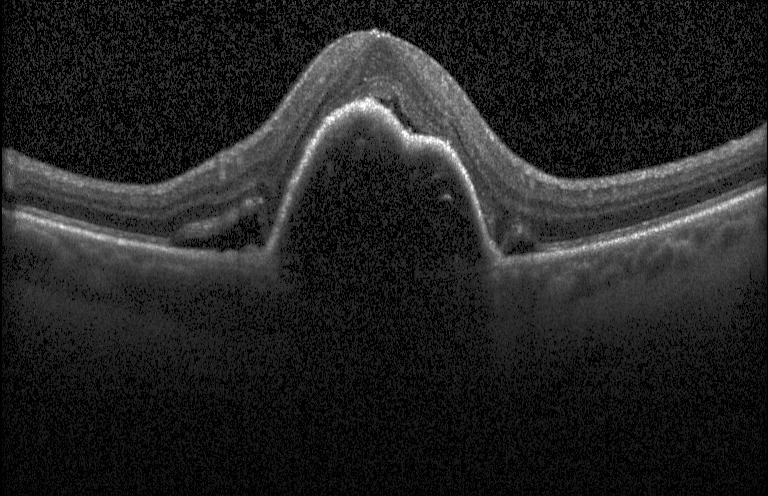
Macular OCT: choroidal neovascularization.